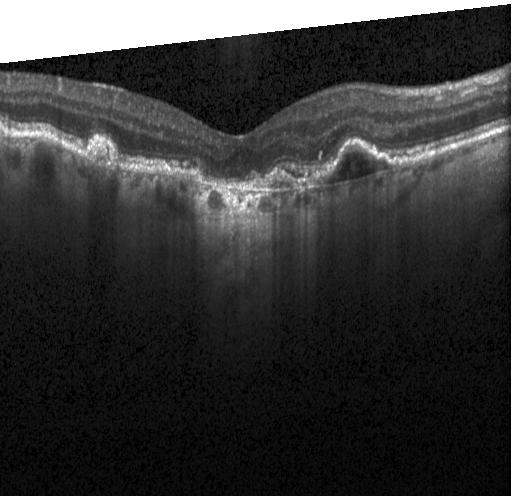

Optical coherence tomography scan
Macular OCT: choroidal neovascularization.